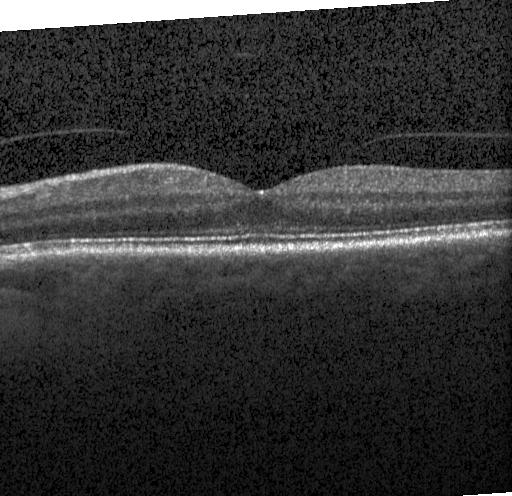 Retinal OCT cross-section, through the macula, Heidelberg Spectralis, spectral-domain optical coherence tomography
Neither choroidal neovascularization, diabetic macular edema, nor drusen.